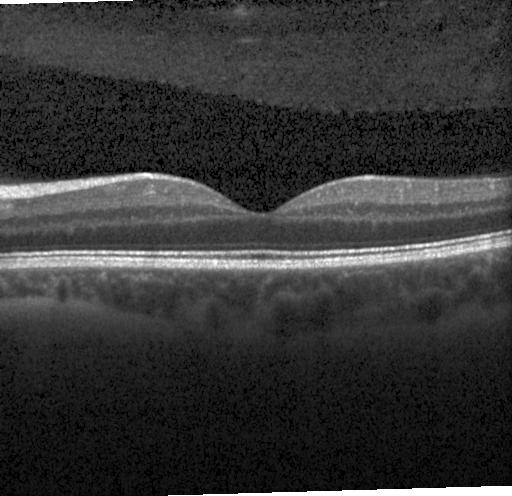 Heidelberg Spectralis OCT system. Optical coherence tomography scan.
Impression: no evidence of CNV, DME, or drusen.